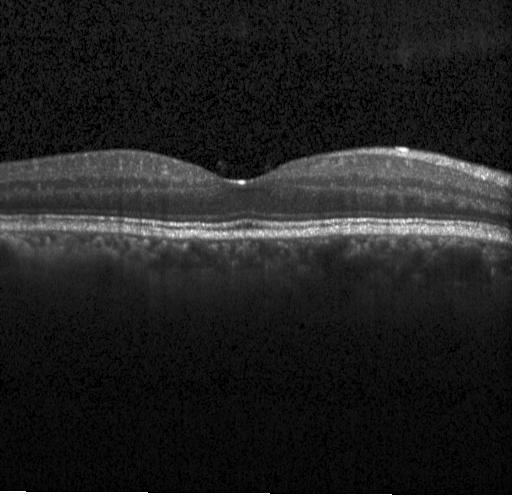

OCT B-scan showing neither CNV, DME, nor drusen.